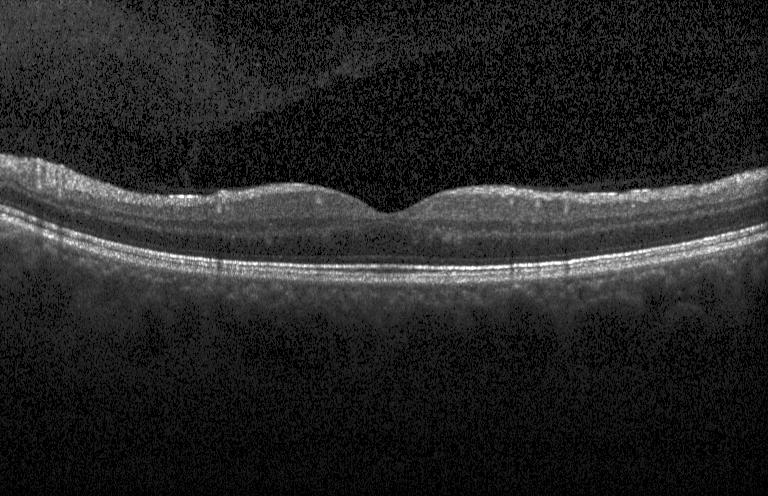

Retinal OCT cross-section
Dx: neither choroidal neovascularization, diabetic macular edema, nor drusen.